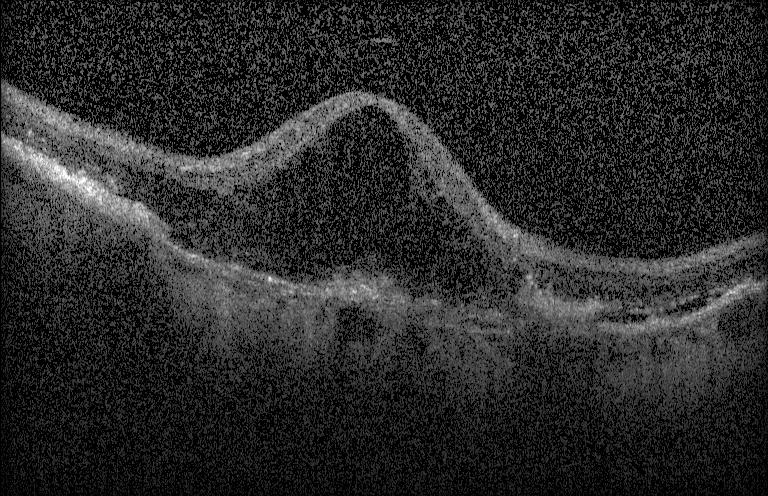

OCT B-scan — This B-scan demonstrates a choroidal neovascular membrane.